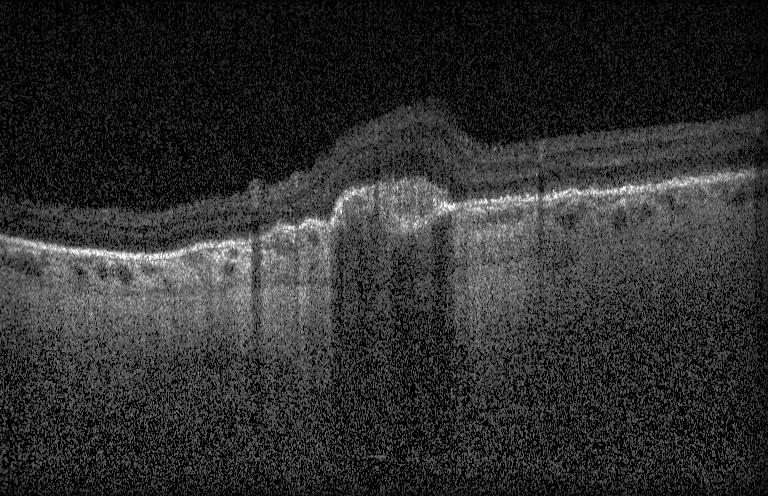

Heidelberg Spectralis; retinal OCT cross-section; SD-OCT.
This B-scan demonstrates a choroidal neovascular membrane.